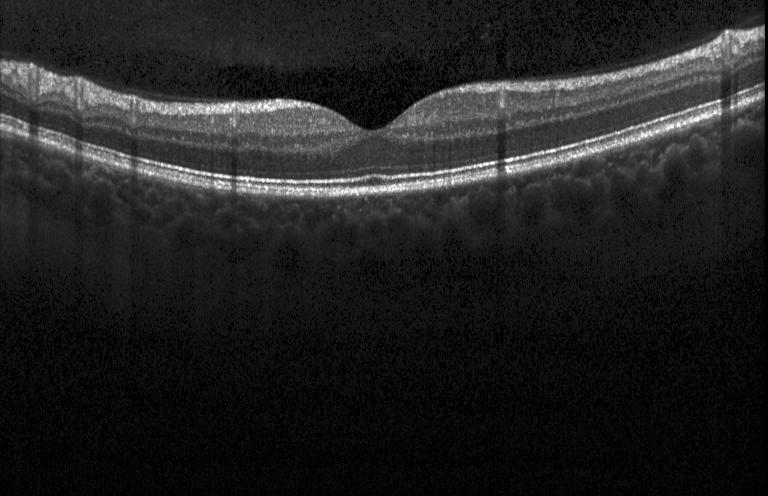 Impression: no evidence of choroidal neovascularization, diabetic macular edema, or drusen.